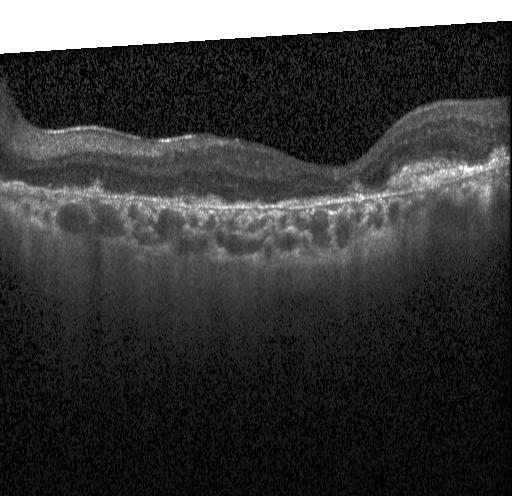
OCT B-scan showing CNV.